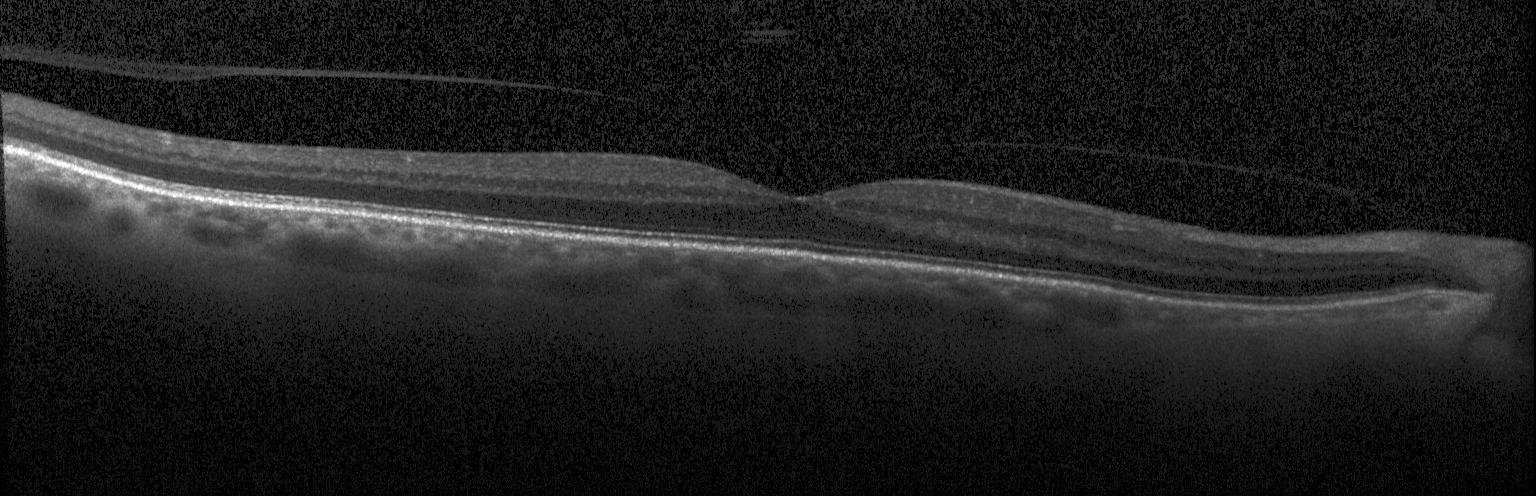
Retinal OCT B-scan
Impression: no choroidal neovascularization, diabetic macular edema, or drusen.